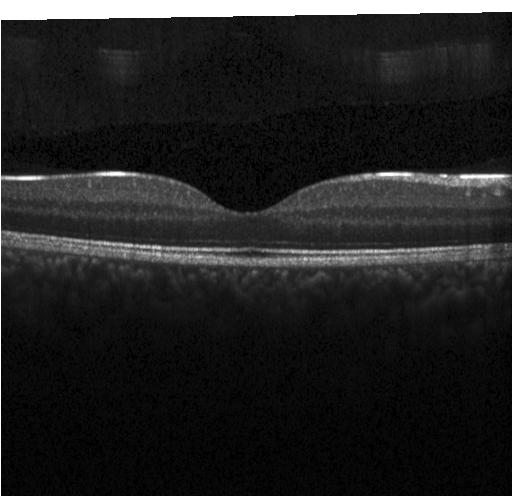
No CNV, no DME, and no drusen.